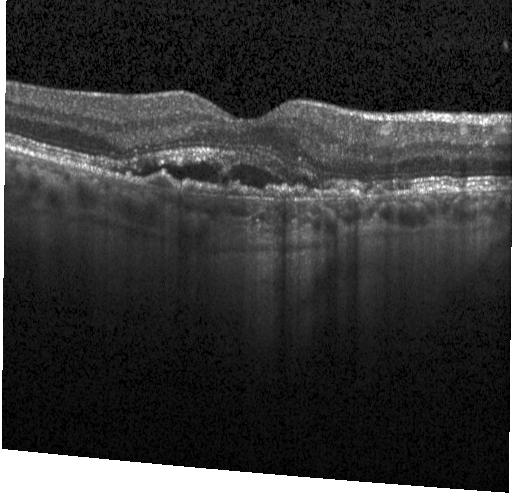

Optical coherence tomography scan — This B-scan demonstrates a choroidal neovascular membrane.